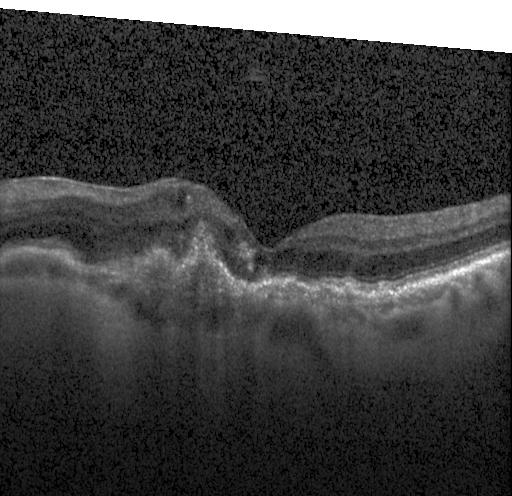 OCT B-scan showing a choroidal neovascular membrane.